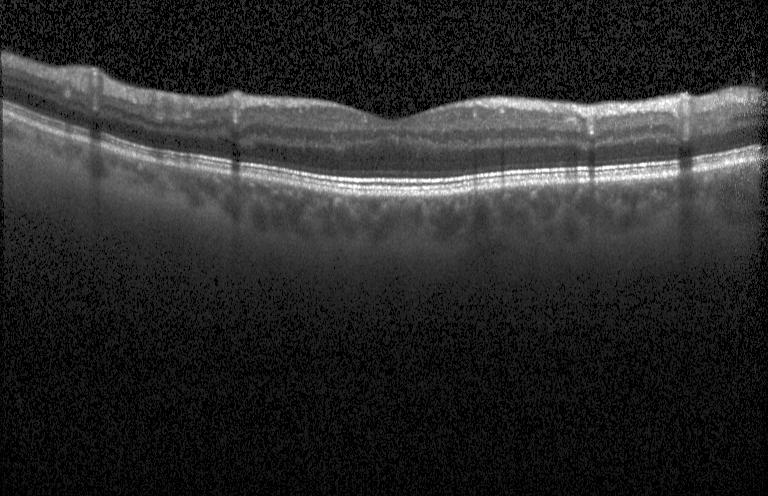
Finding: no evidence of CNV, DME, or drusen.